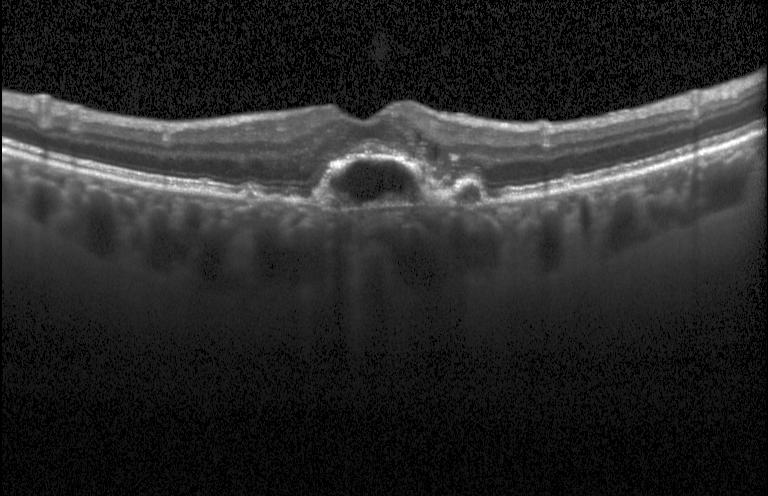
Diagnosis: a choroidal neovascular membrane.